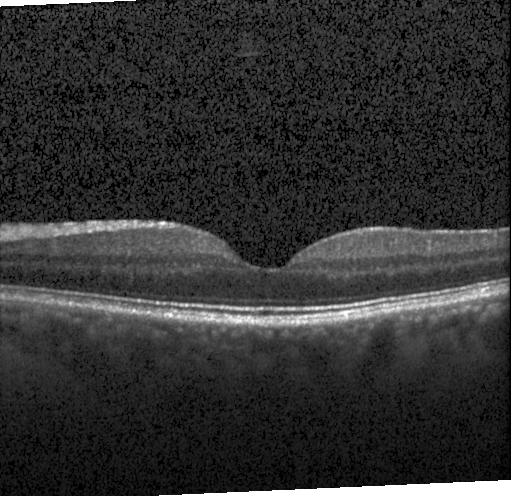
OCT line scan. Instrument: Heidelberg Spectralis. SD-OCT
Diagnosis: no choroidal neovascularization, no diabetic macular edema, and no drusen.